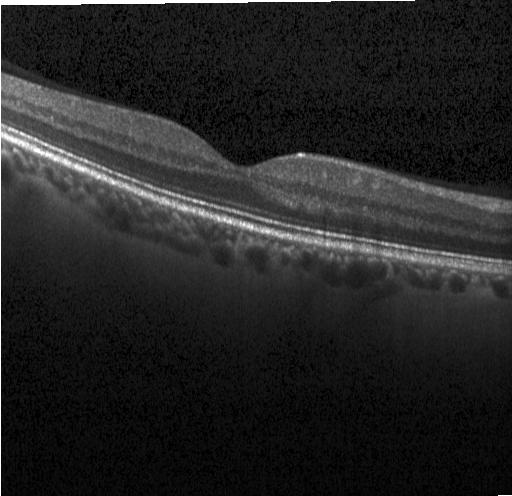
The scan shows no choroidal neovascularization, diabetic macular edema, or drusen.